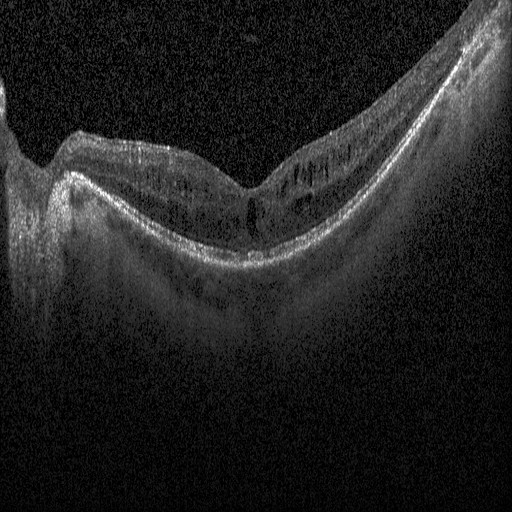 Assessment: diabetic macular edema (DME).